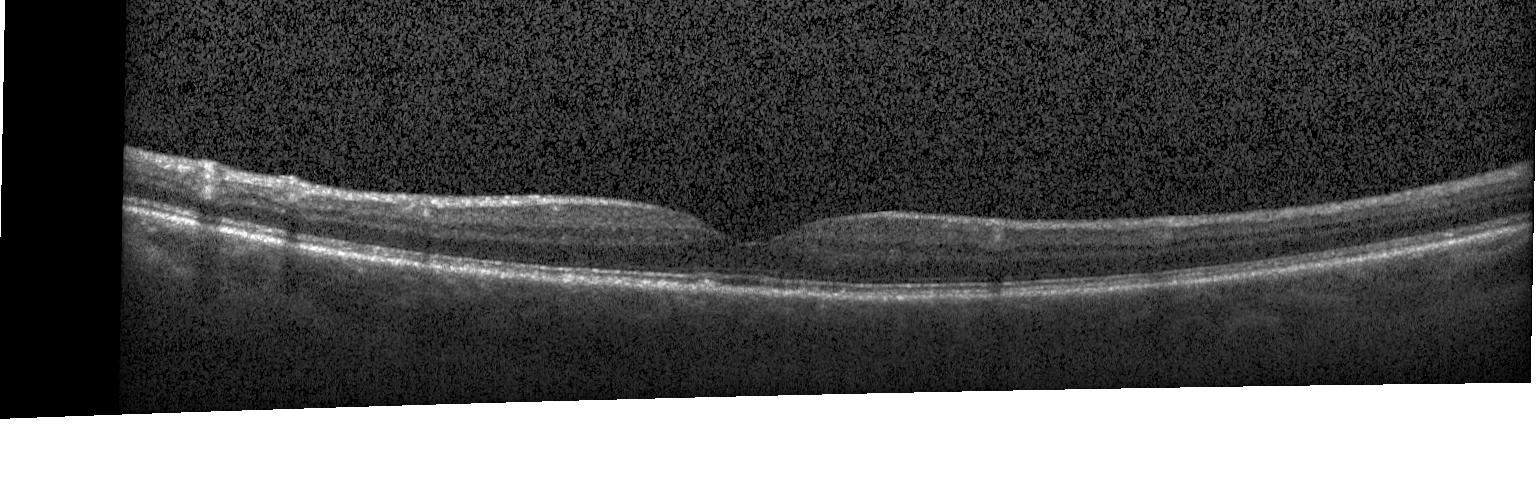

OCT B-scan showing no choroidal neovascularization, diabetic macular edema, or drusen.